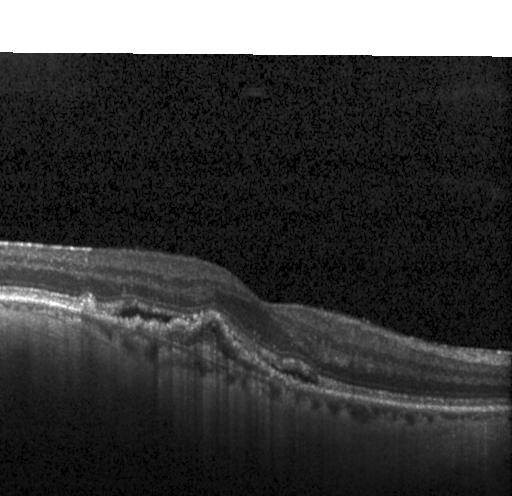 Macular OCT demonstrating CNV.